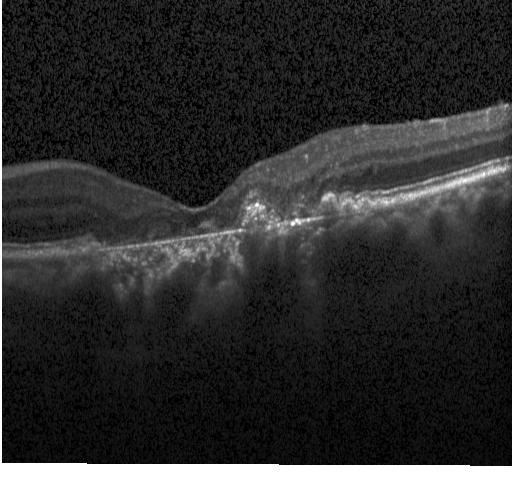 Dx: choroidal neovascularization (CNV).